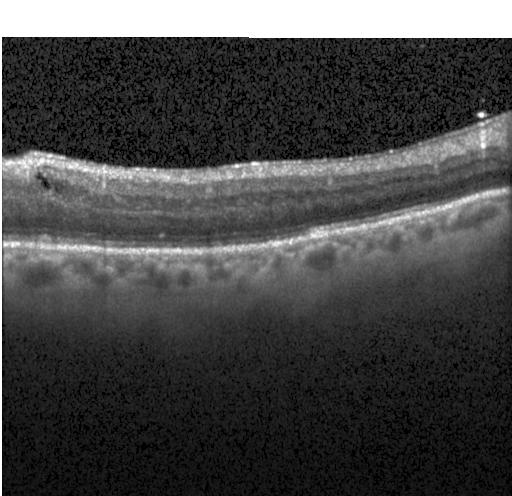
Assessment: DME.